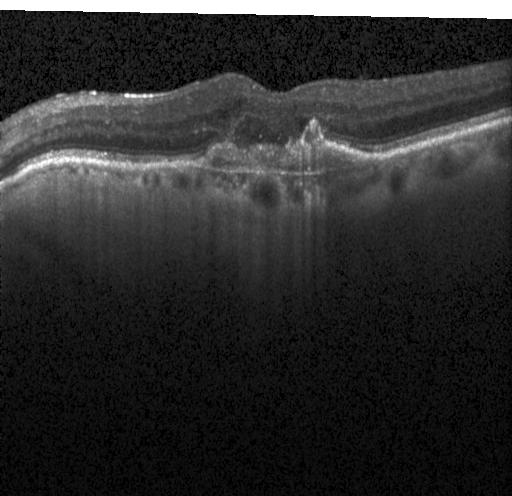

Spectral-domain optical coherence tomography, optical coherence tomography scan
This B-scan demonstrates choroidal neovascularization.